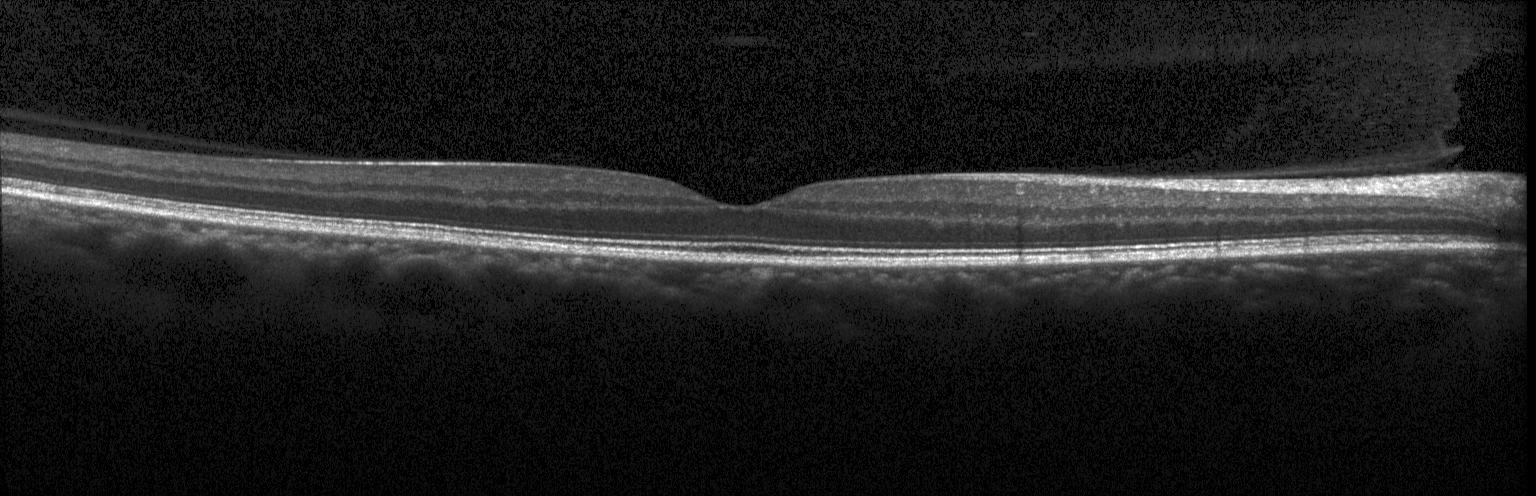
OCT scan showing no CNV, no DME, and no drusen.